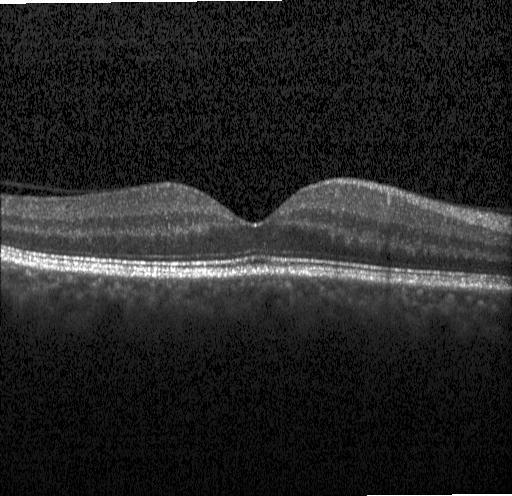 Impression: neither choroidal neovascularization, diabetic macular edema, nor drusen.